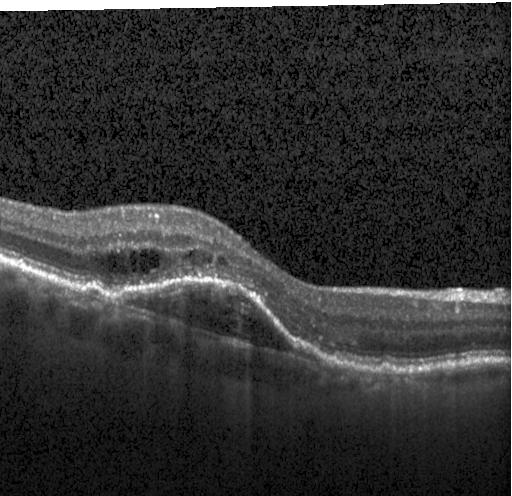

Retinal OCT B-scan. A choroidal neovascular membrane.